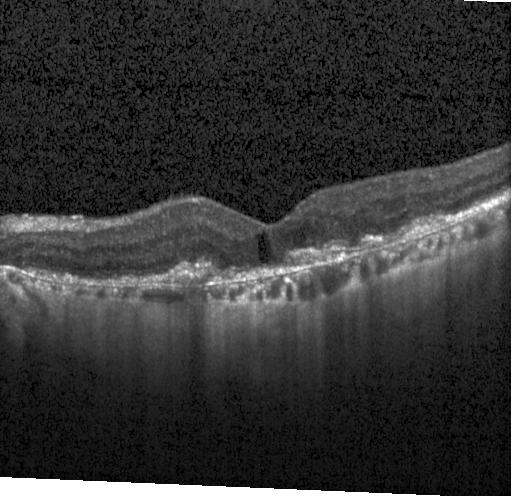 SD-OCT. Heidelberg Spectralis. Horizontal scan through the fovea. OCT line scan. Assessment: choroidal neovascularization.